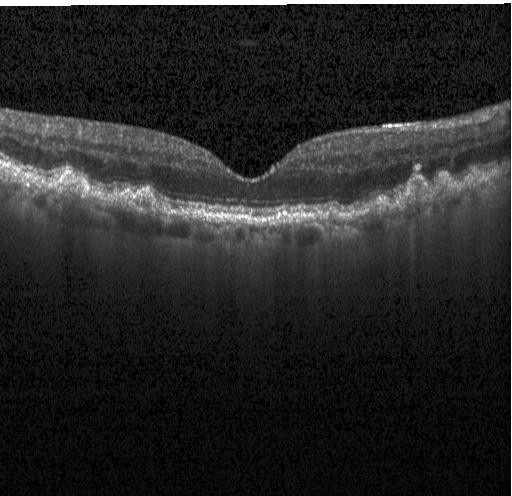

Through the macula, SD-OCT, retinal OCT B-scan — Dx: drusen.